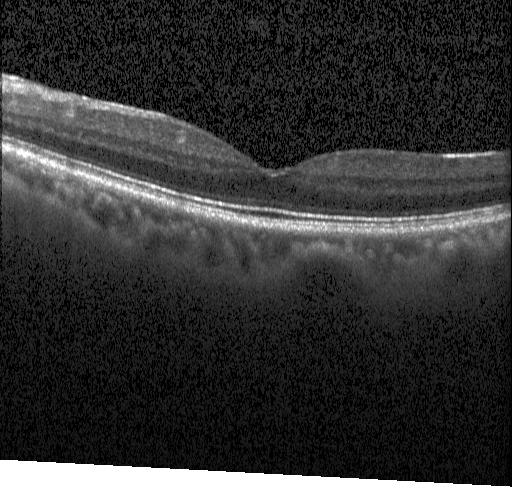

Dx: neither CNV, DME, nor drusen.